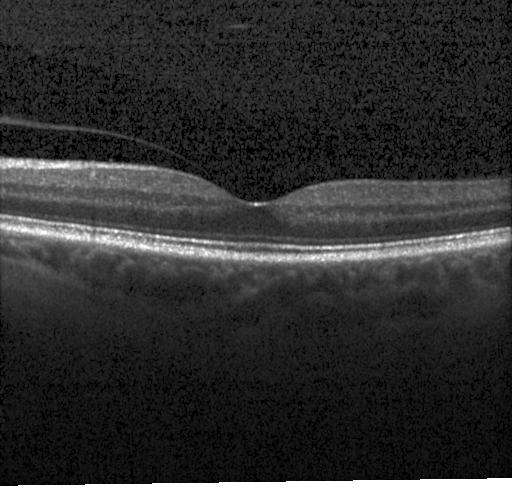

Assessment: neither choroidal neovascularization, diabetic macular edema, nor drusen.